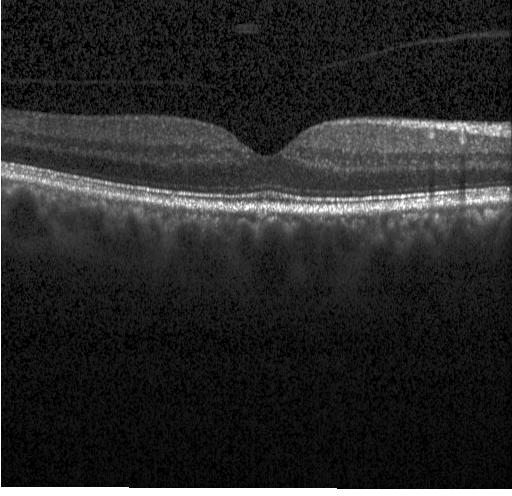 Acquired on a Heidelberg Spectralis; retinal OCT B-scan.
The scan shows neither choroidal neovascularization, diabetic macular edema, nor drusen.